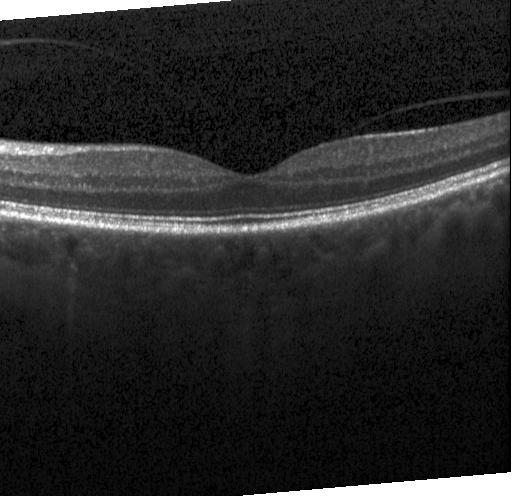 OCT line scan; SD-OCT; instrument: Heidelberg Spectralis; horizontal scan through the fovea — Impression: no CNV, no DME, and no drusen.